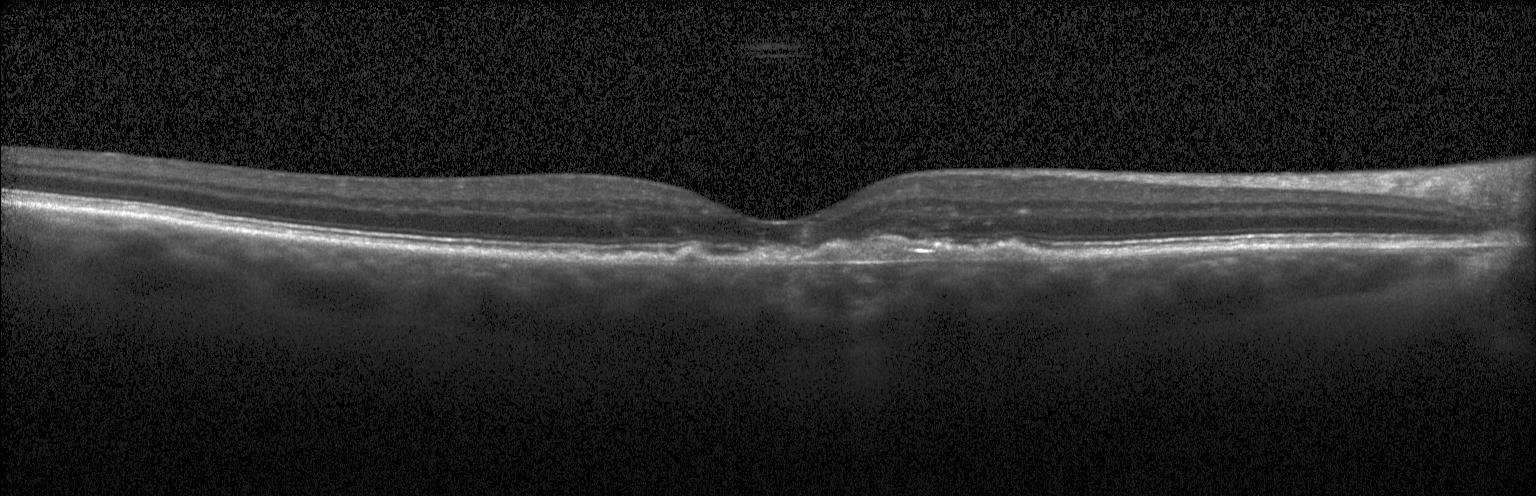

Optical coherence tomography scan. Spectral-domain optical coherence tomography. Diagnosis: choroidal neovascularization (CNV).